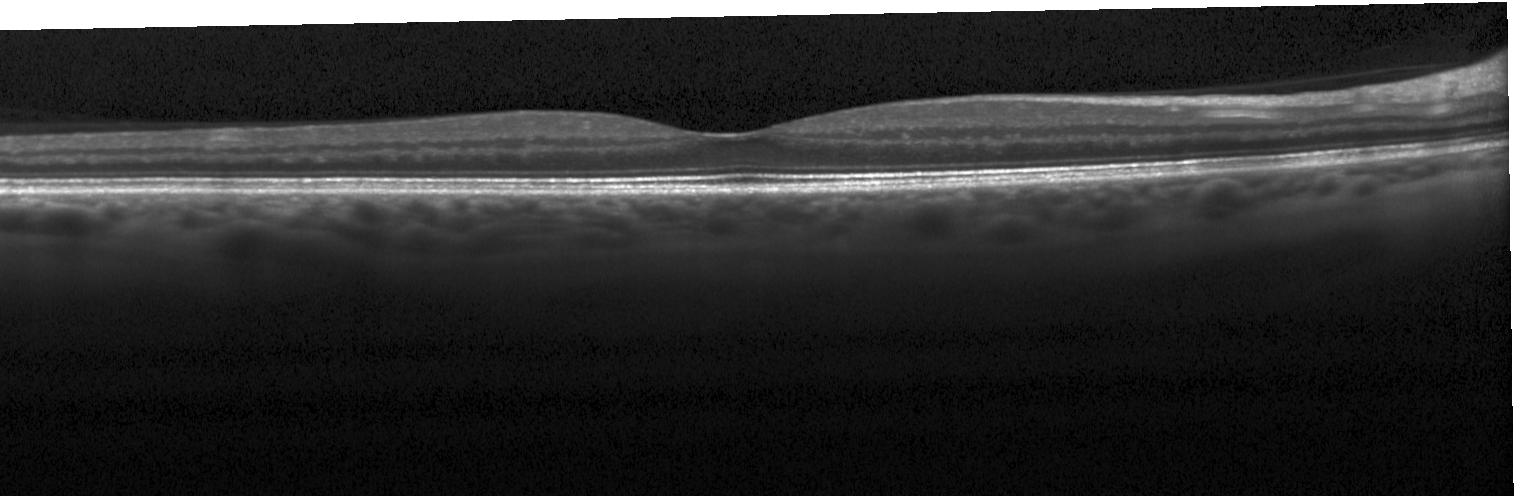
Retinal OCT cross-section, horizontal scan through the fovea, Heidelberg Spectralis OCT system. Dx: no choroidal neovascularization, no diabetic macular edema, and no drusen.